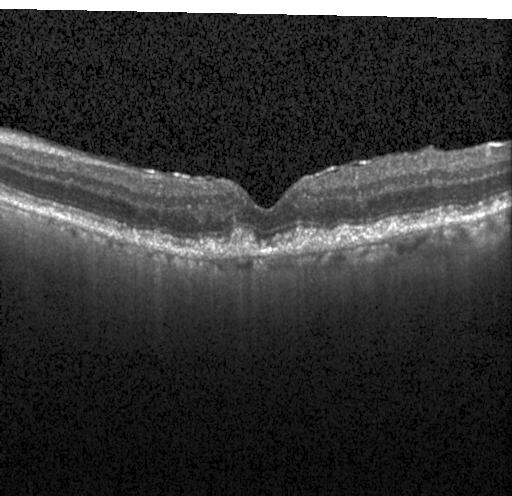

OCT B-scan · SD-OCT
OCT finding: multiple drusen.